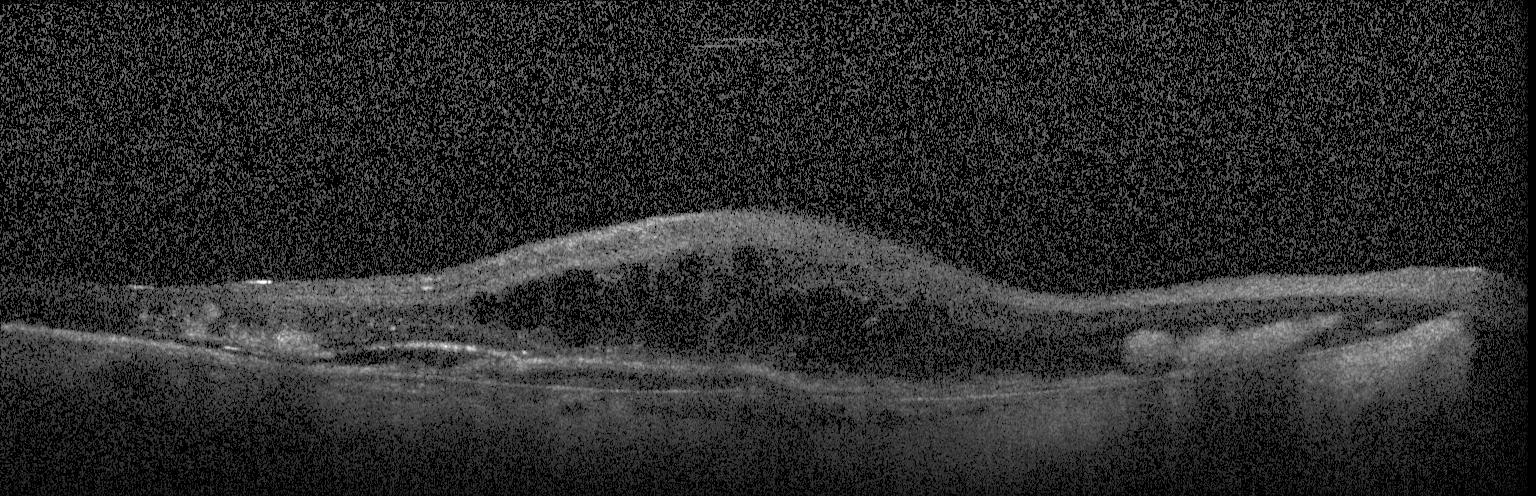 OCT finding: choroidal neovascularization (CNV).